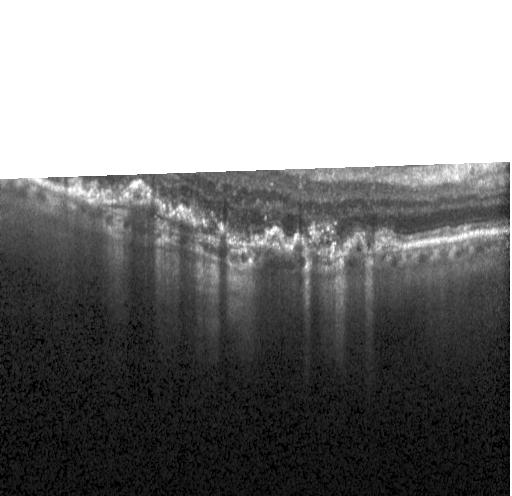
Dx: a choroidal neovascular membrane.